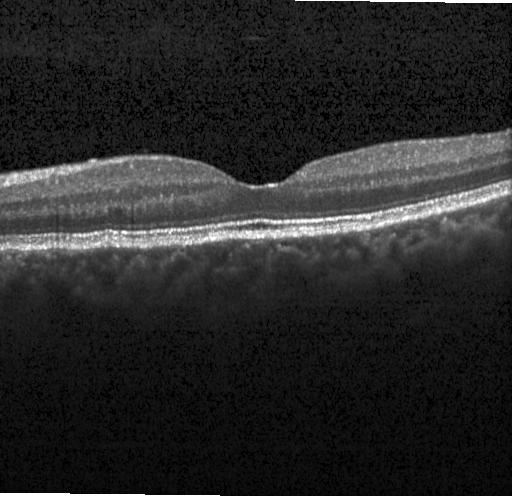 Macular OCT: no evidence of CNV, DME, or drusen.